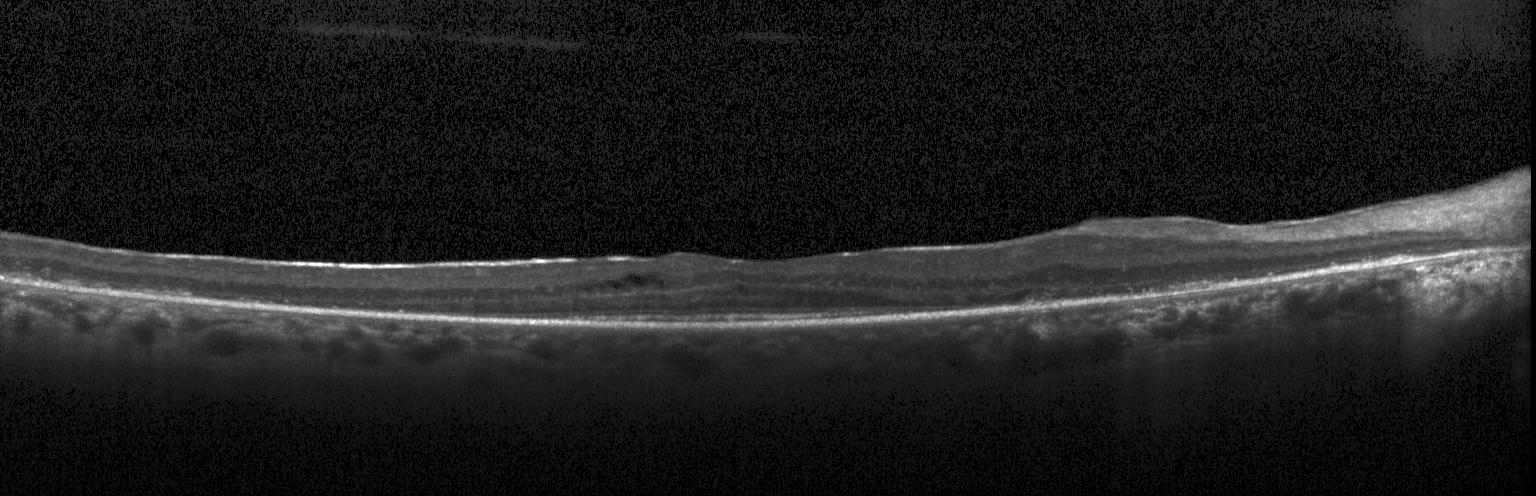
OCT scan showing DME.